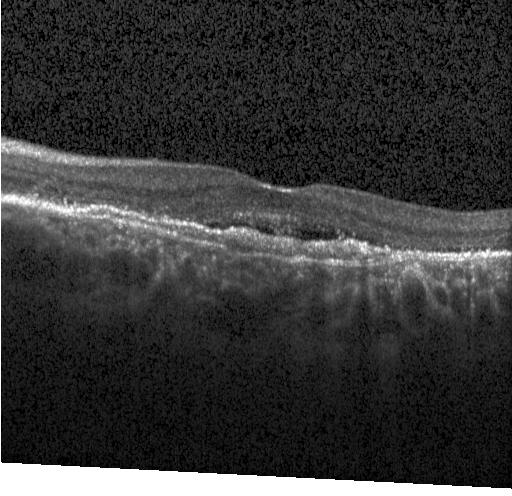 OCT line scan — Impression: a choroidal neovascular membrane.